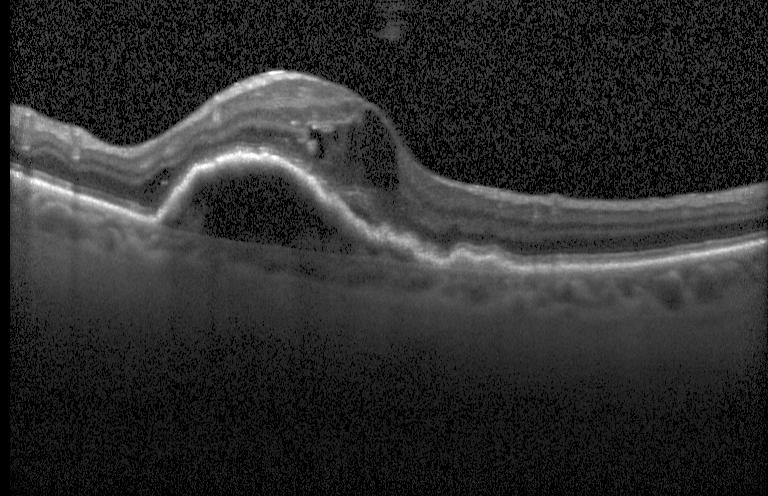 OCT B-scan; spectral-domain optical coherence tomography; Heidelberg Spectralis.
This B-scan demonstrates a choroidal neovascular membrane.